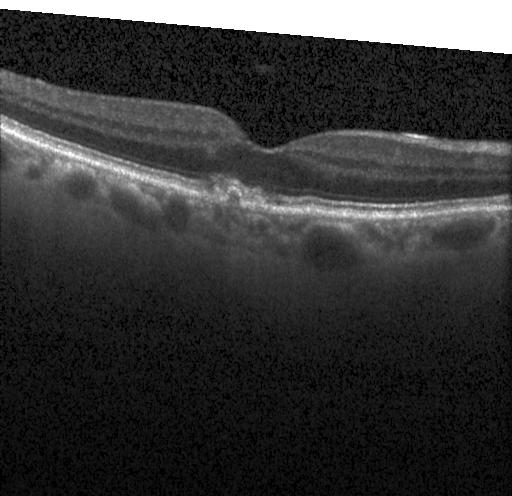
Finding: a choroidal neovascular membrane.